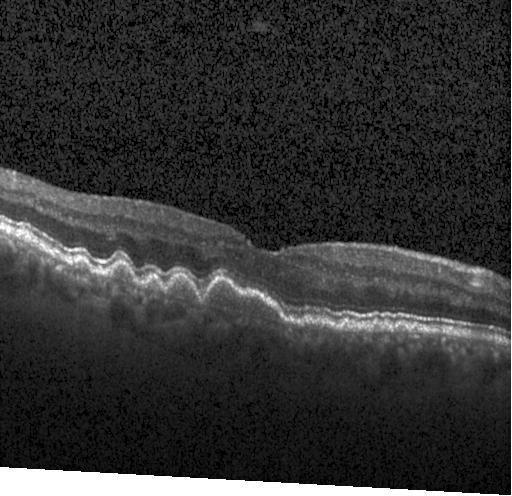

Finding: drusen.